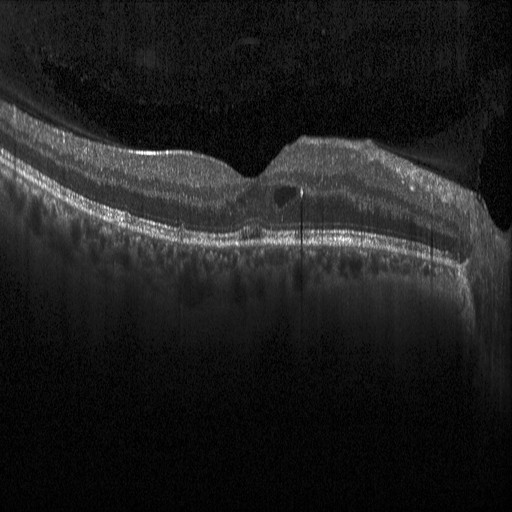
Optical coherence tomography B-scan. Diagnosis: DME.